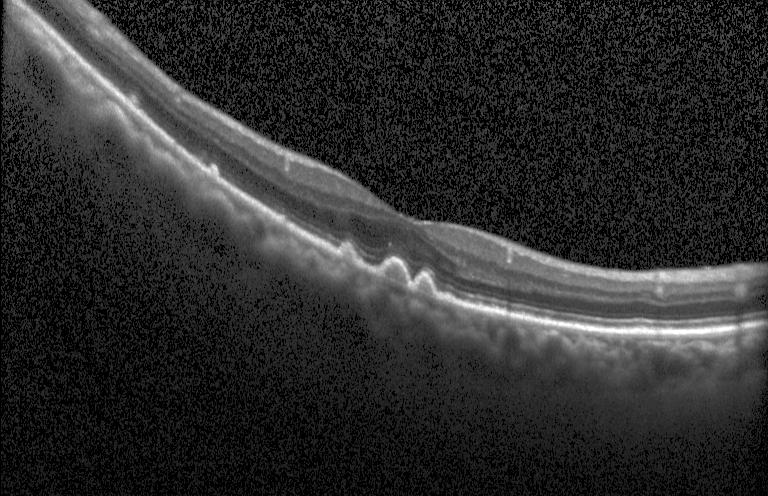 Retinal OCT B-scan · spectral-domain OCT. This B-scan demonstrates drusen.